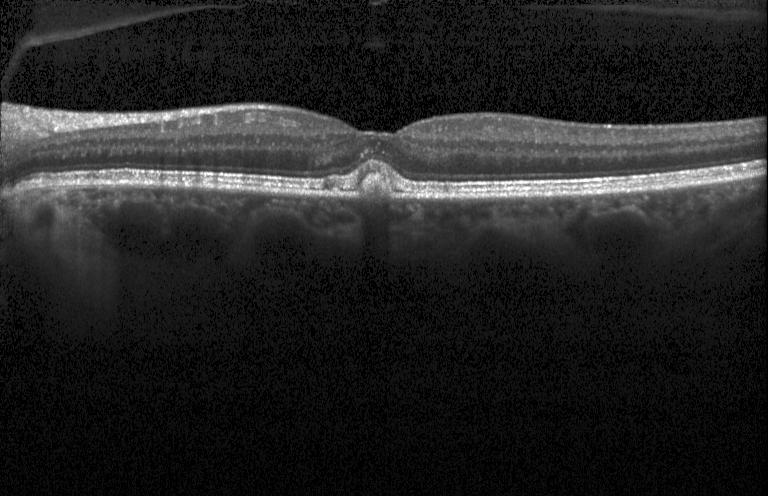 Assessment: sub-RPE drusenoid deposits.